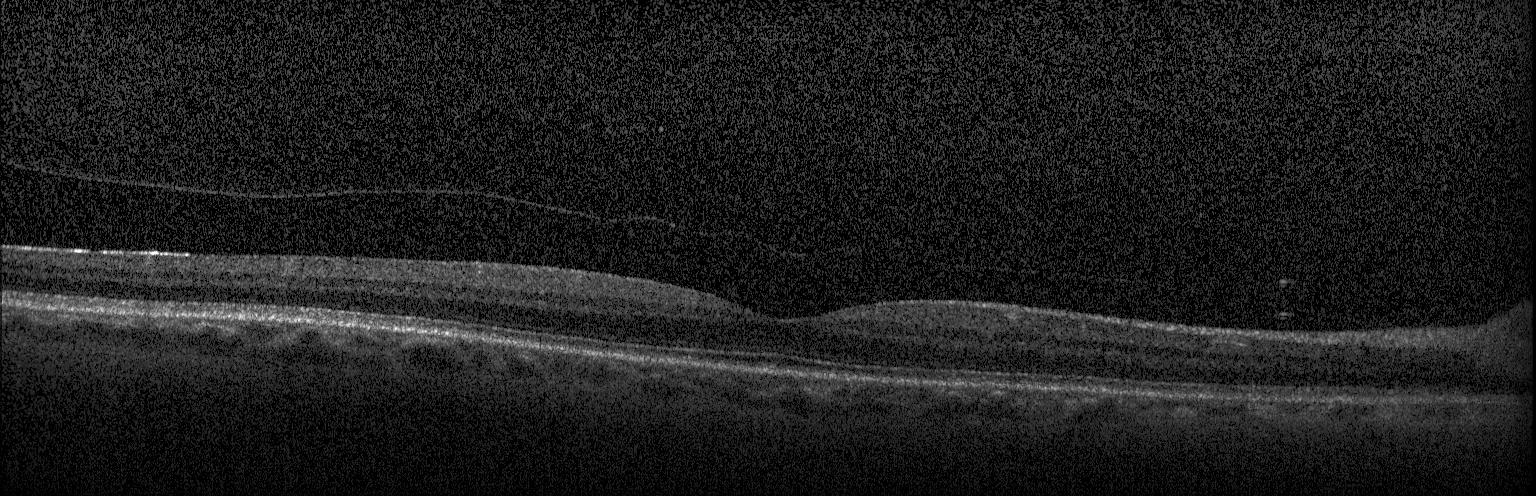 OCT B-scan.
Impression: no choroidal neovascularization, no diabetic macular edema, and no drusen.